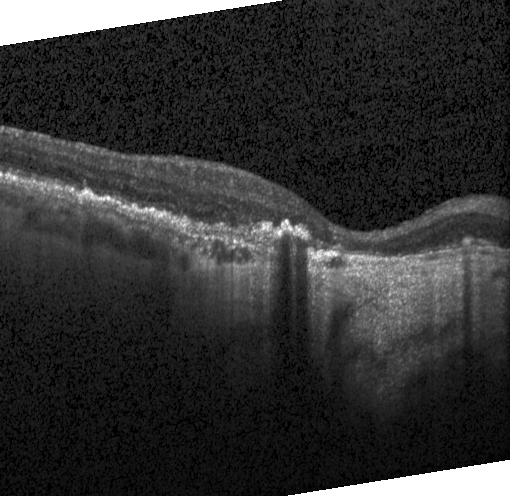
Assessment: a choroidal neovascular membrane.